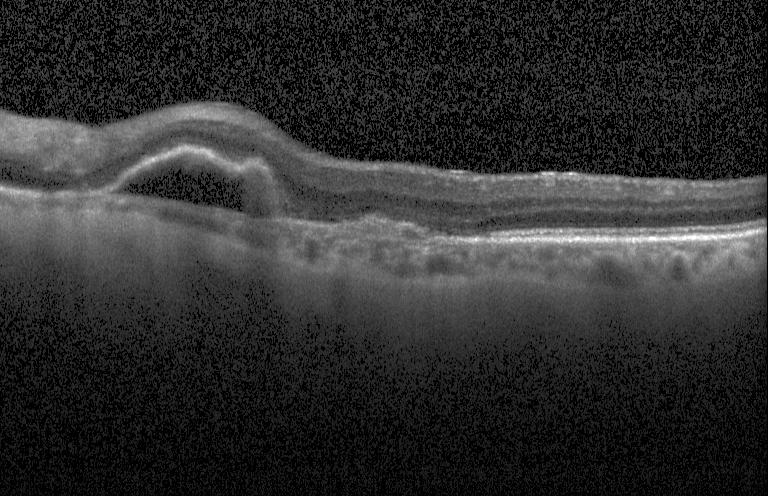

OCT B-scan; fovea-centered; spectral-domain optical coherence tomography — Finding: a choroidal neovascular membrane.